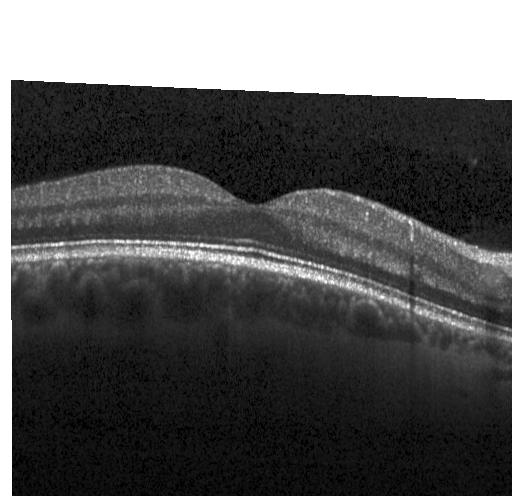
Impression: neither choroidal neovascularization, diabetic macular edema, nor drusen.